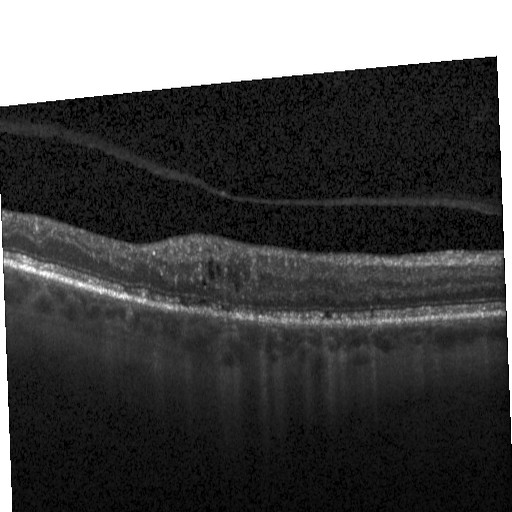

OCT scan showing DME.